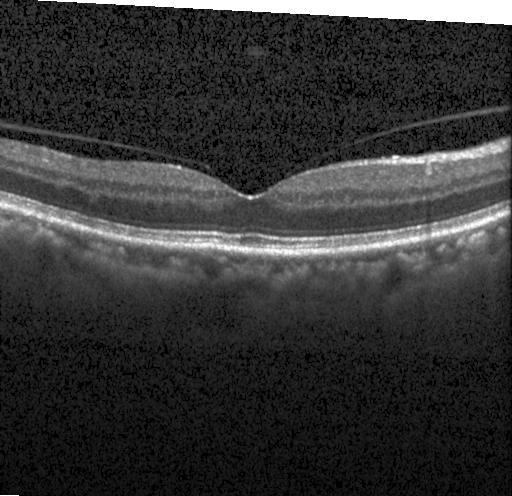

Finding: neither CNV, DME, nor drusen.